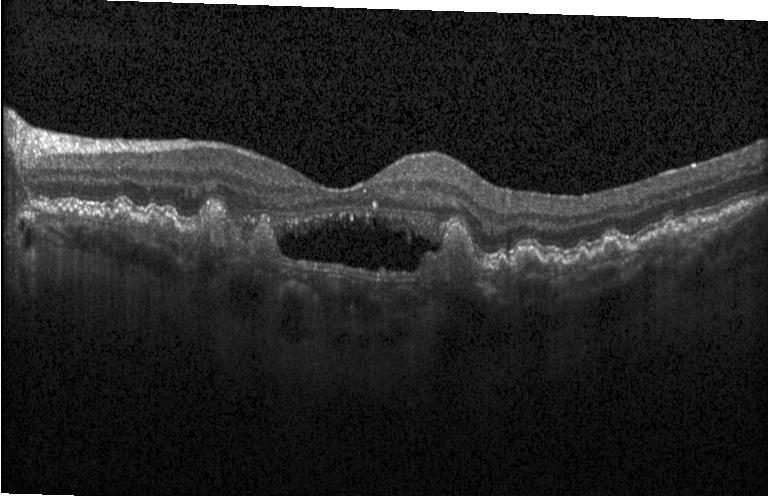
Finding: a choroidal neovascular membrane.